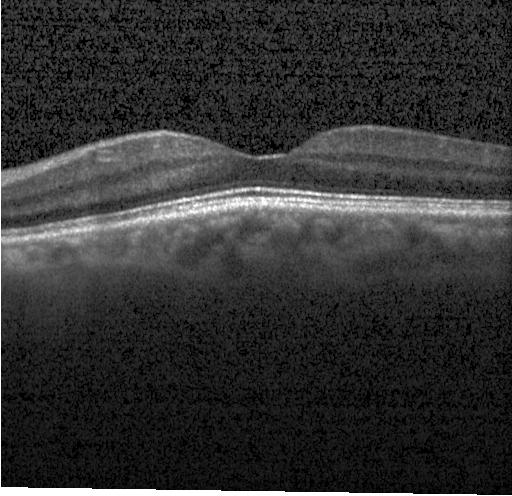

OCT line scan
Finding: no CNV, DME, or drusen.